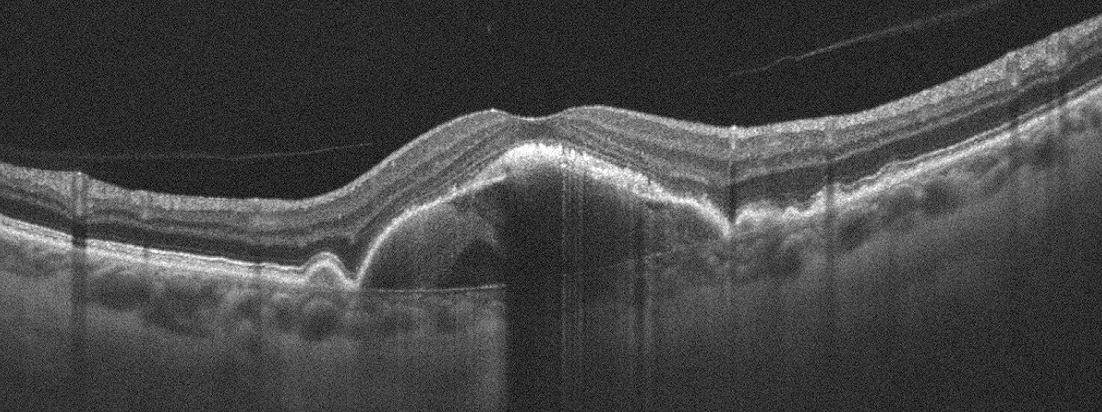

Retinal OCT B-scan · Optovue Avanti RTVue XR
Finding: age-related macular degeneration.